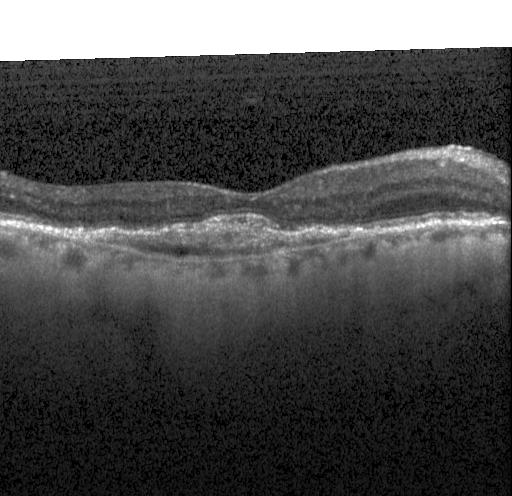 Optical coherence tomography B-scan — The scan shows a choroidal neovascular membrane.